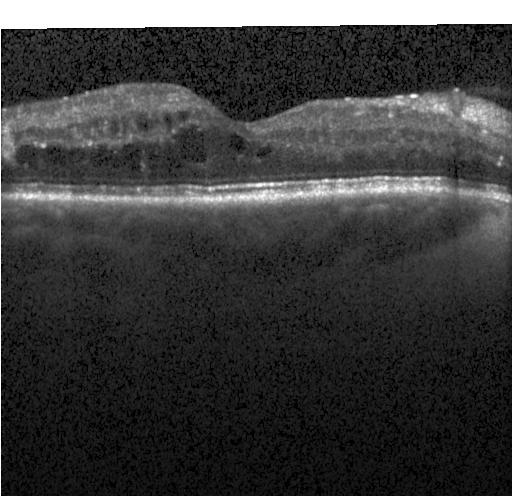
Macular scan · OCT line scan — Diagnosis: DME.